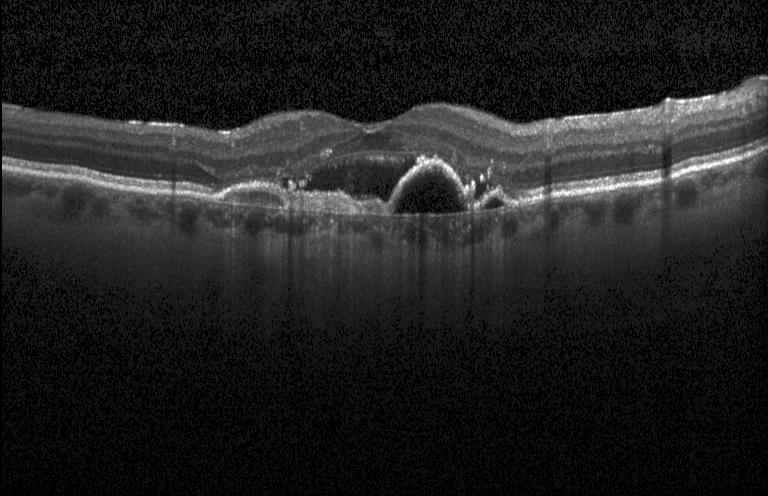 Macular OCT: CNV.